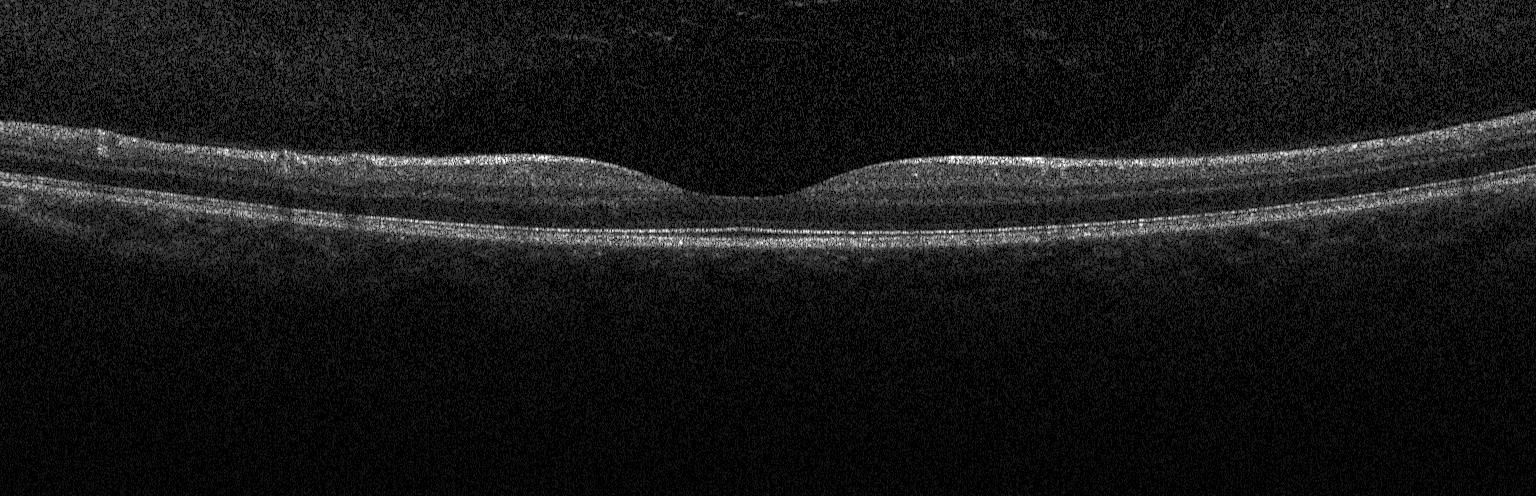 OCT line scan
Impression: no evidence of choroidal neovascularization, diabetic macular edema, or drusen.